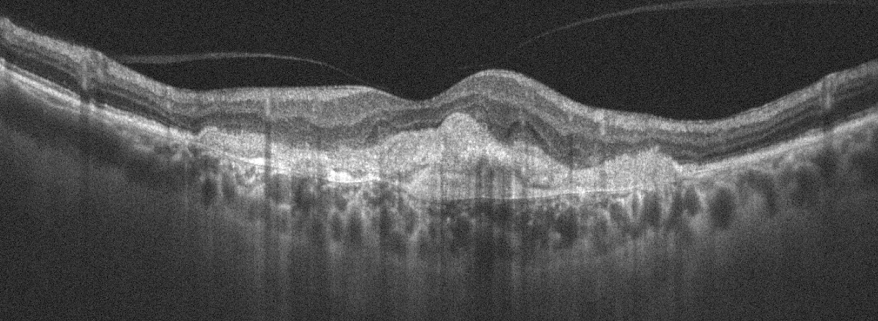
Impression: age-related macular degeneration.